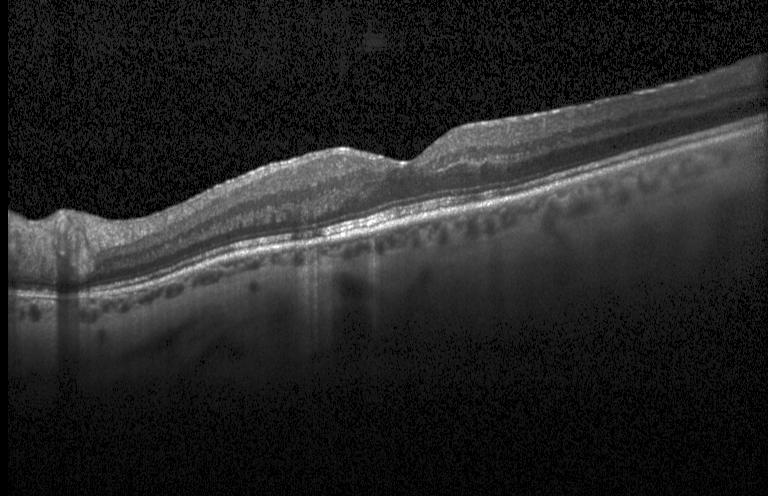
Horizontal scan through the fovea; spectral-domain optical coherence tomography; optical coherence tomography B-scan. Macular OCT: neither choroidal neovascularization, diabetic macular edema, nor drusen.